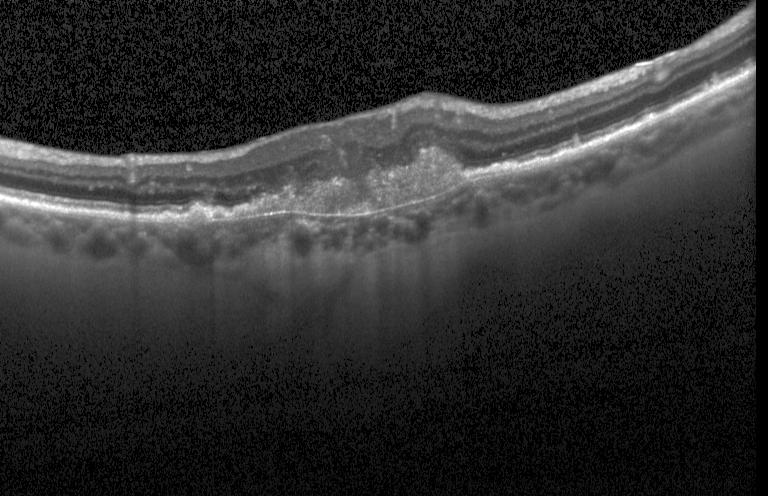

Retinal OCT B-scan.
Finding: choroidal neovascularization (CNV).